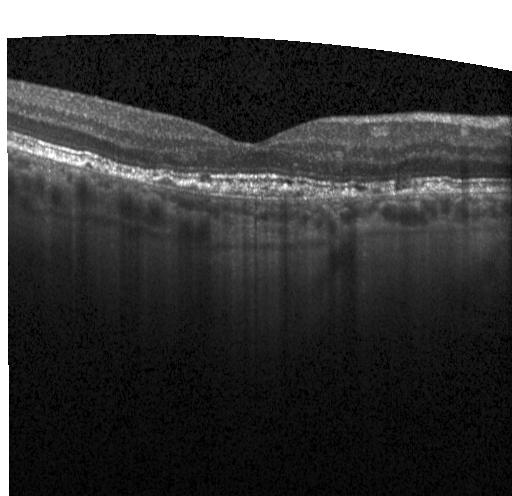 Dx: choroidal neovascularization.